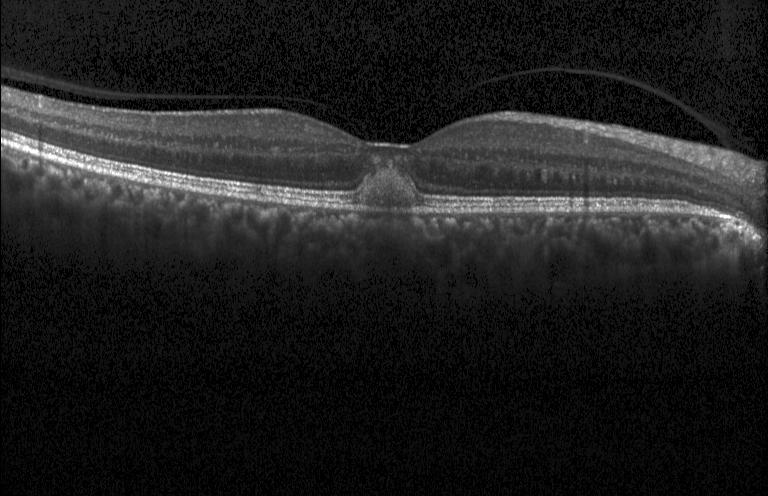
Impression: a choroidal neovascular membrane.